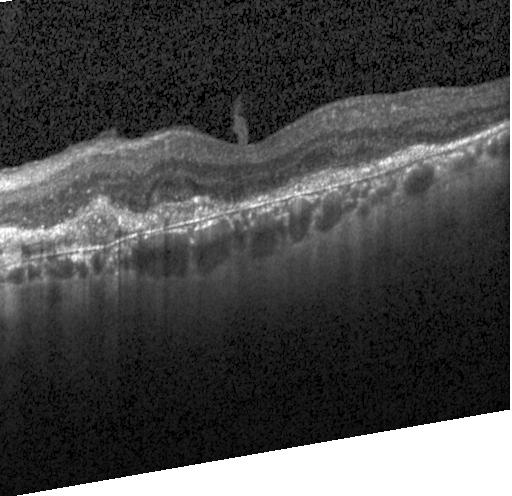 Acquired on a Heidelberg Spectralis, SD-OCT, OCT line scan — Assessment: choroidal neovascularization.